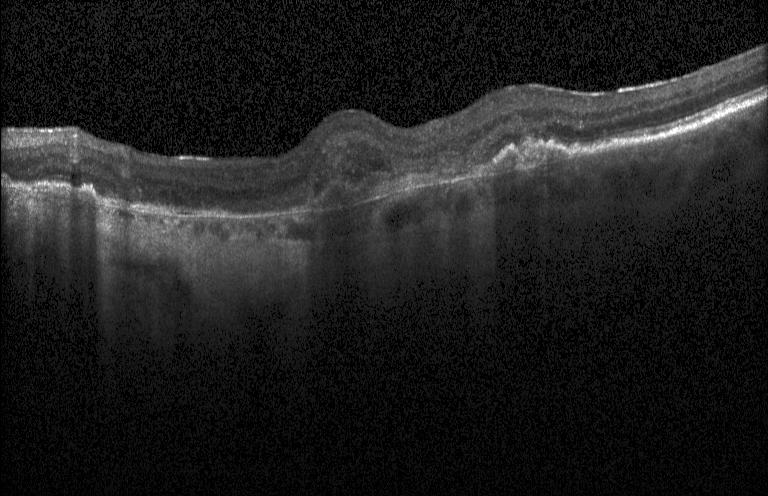 Spectral-domain optical coherence tomography · OCT line scan · acquired on a Heidelberg Spectralis · macular scan — Assessment: a choroidal neovascular membrane.